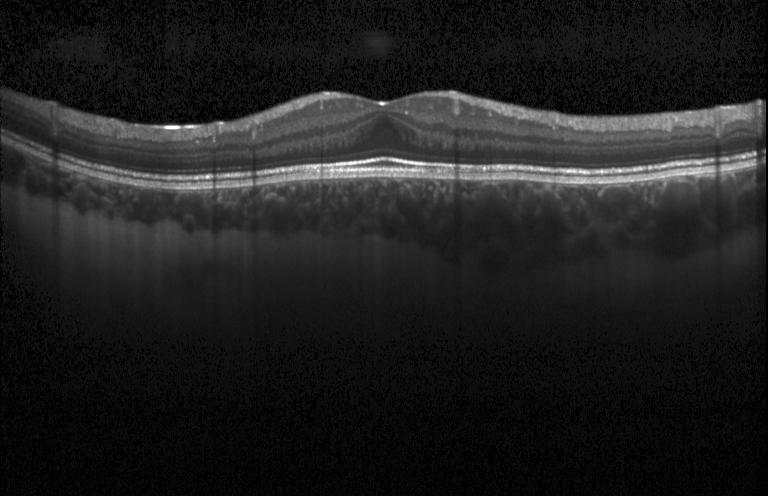

Macular scan; Heidelberg Spectralis OCT system; spectral-domain optical coherence tomography; retinal OCT B-scan
Diagnosis: no evidence of choroidal neovascularization, diabetic macular edema, or drusen.